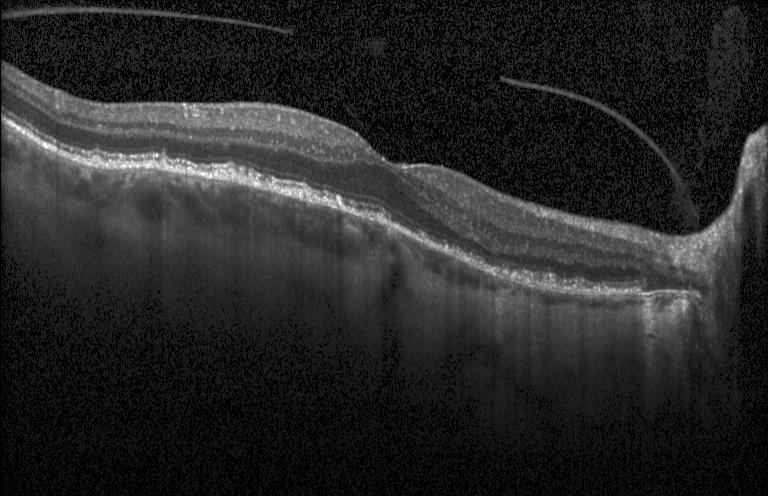
Optical coherence tomography B-scan; horizontal scan through the fovea; Heidelberg Spectralis OCT system.
This B-scan demonstrates drusen.